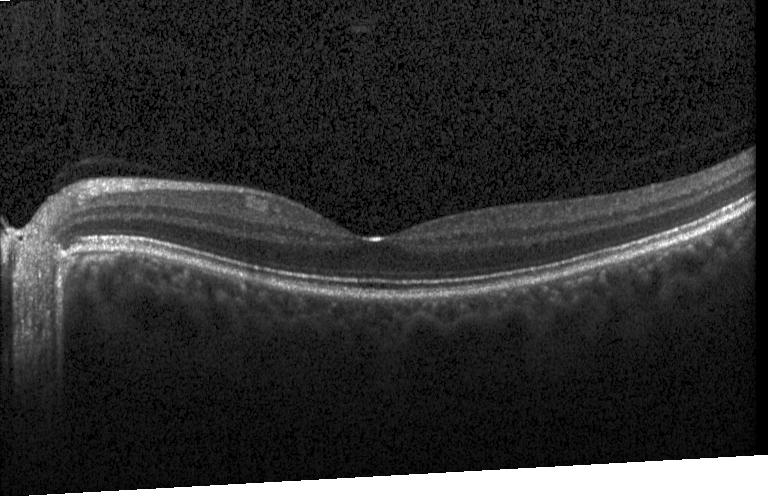

Assessment: no CNV, DME, or drusen.